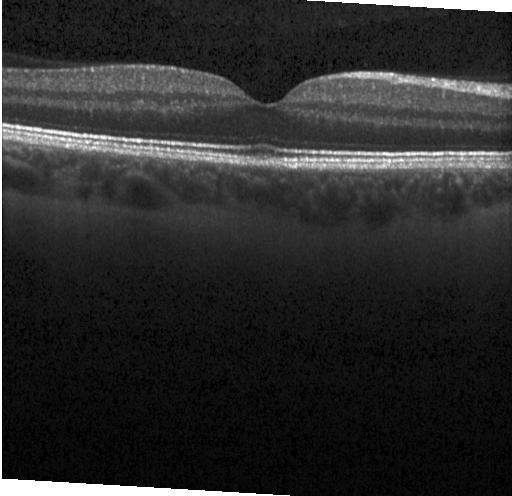 Diagnosis: no choroidal neovascularization, diabetic macular edema, or drusen.